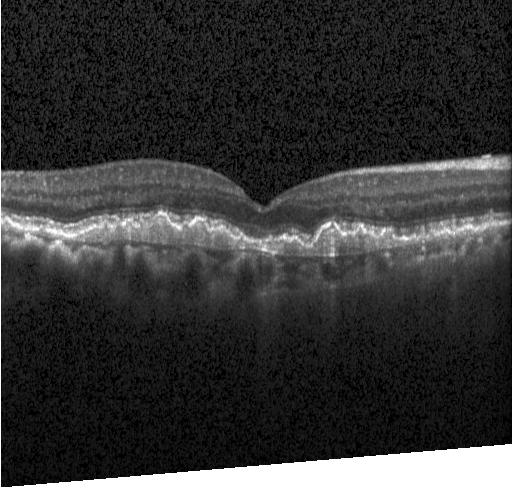
Macular OCT demonstrating a choroidal neovascular membrane.